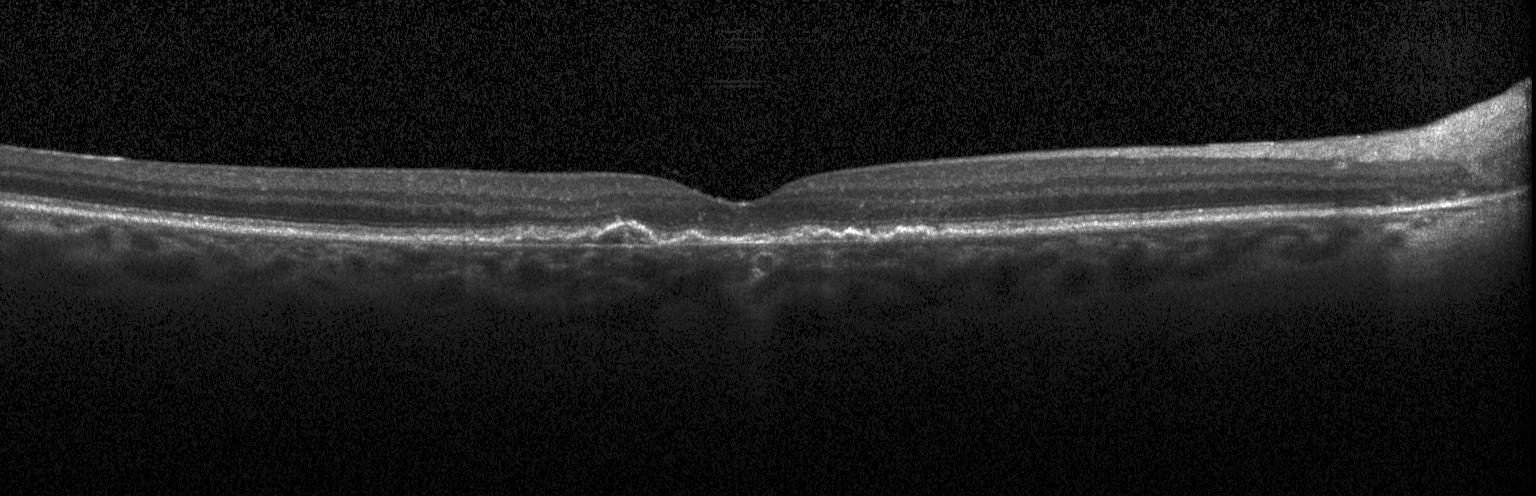

Optical coherence tomography B-scan · fovea-centered. Finding: a choroidal neovascular membrane.